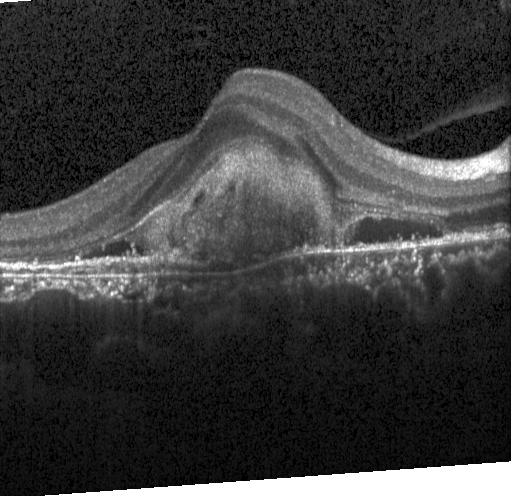 OCT B-scan. The scan shows a choroidal neovascular membrane.